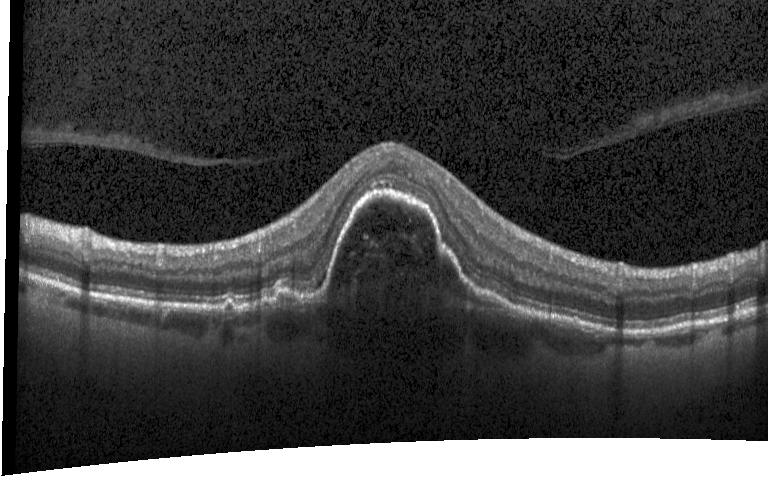

Optical coherence tomography scan; spectral-domain optical coherence tomography — Macular OCT: choroidal neovascularization (CNV).